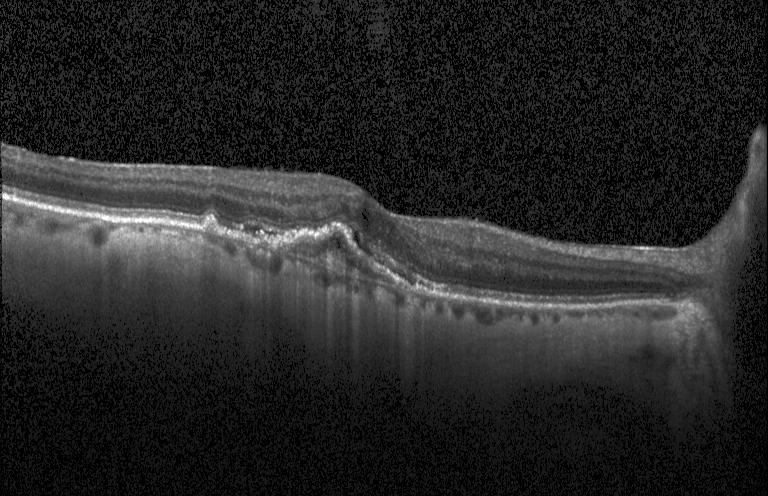

Finding: a choroidal neovascular membrane.